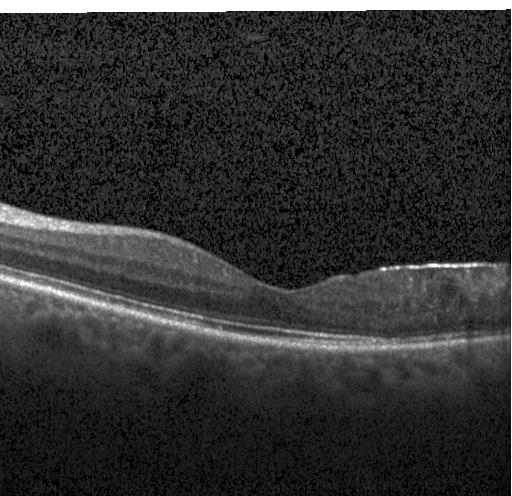

This B-scan demonstrates DME.